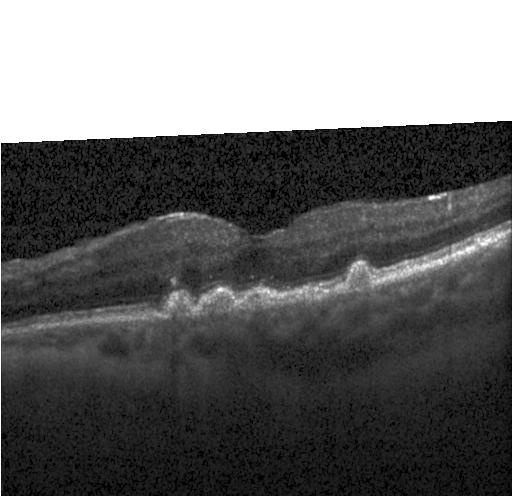 Dx: drusen.